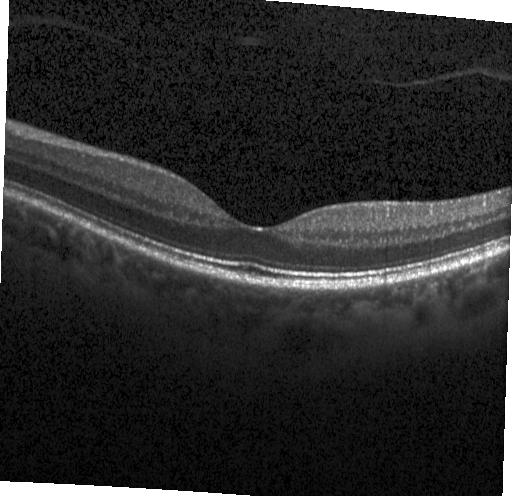
OCT line scan.
Dx: no evidence of CNV, DME, or drusen.